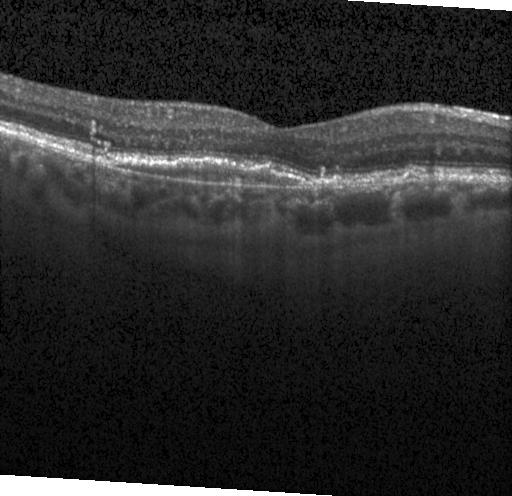
OCT line scan, through the macula, acquired on a Heidelberg Spectralis, spectral-domain OCT. OCT finding: a choroidal neovascular membrane.